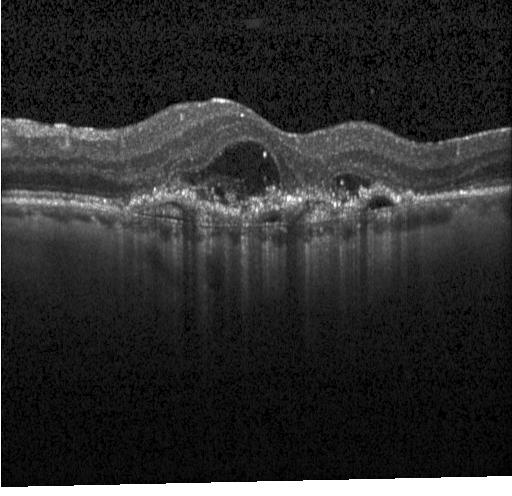

Acquired on a Heidelberg Spectralis. OCT line scan
Impression: a choroidal neovascular membrane.